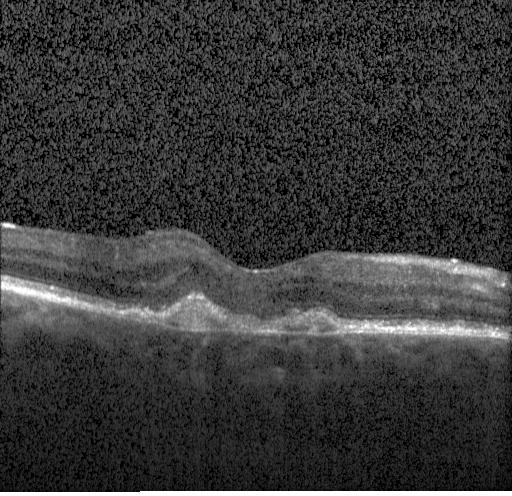
Optical coherence tomography B-scan. Acquired on a Heidelberg Spectralis — Macular OCT: a choroidal neovascular membrane.